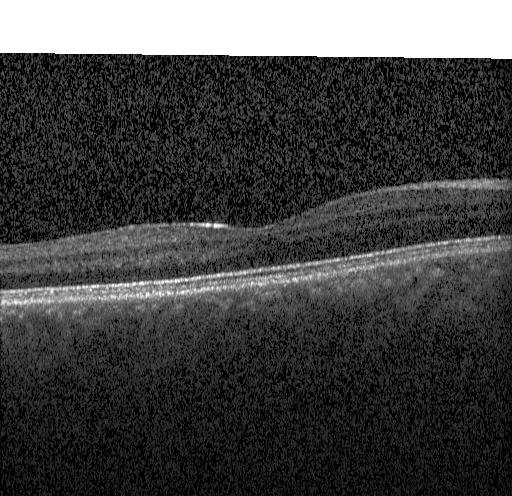 Diagnosis: no CNV, no DME, and no drusen.